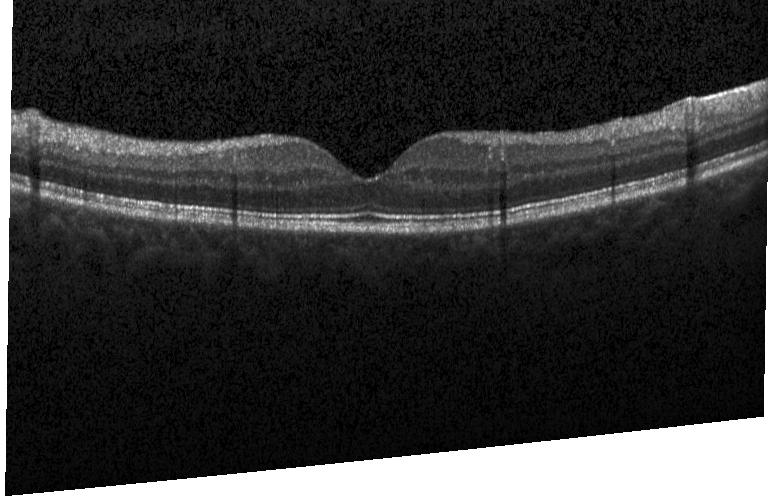

Optical coherence tomography scan — Macular OCT: neither choroidal neovascularization, diabetic macular edema, nor drusen.